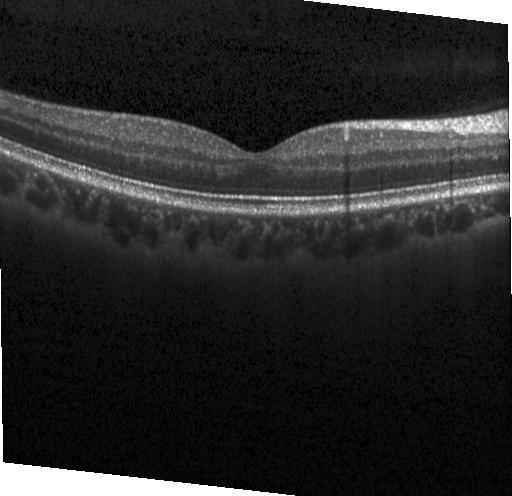

Finding: neither choroidal neovascularization, diabetic macular edema, nor drusen.